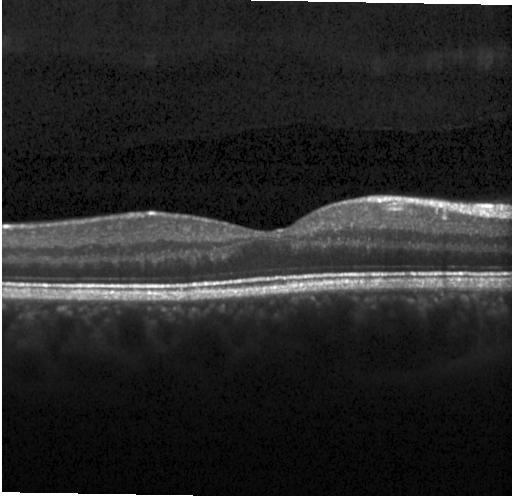 Macular OCT: no choroidal neovascularization, no diabetic macular edema, and no drusen.